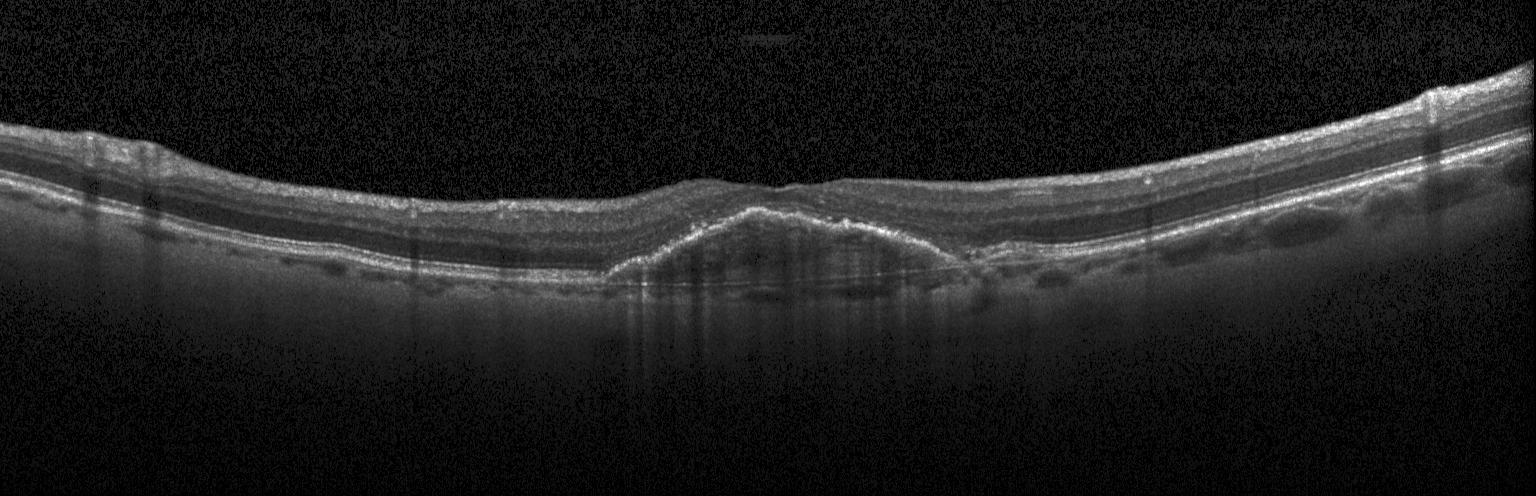

Through the macula; optical coherence tomography scan; instrument: Heidelberg Spectralis.
OCT finding: choroidal neovascularization (CNV).